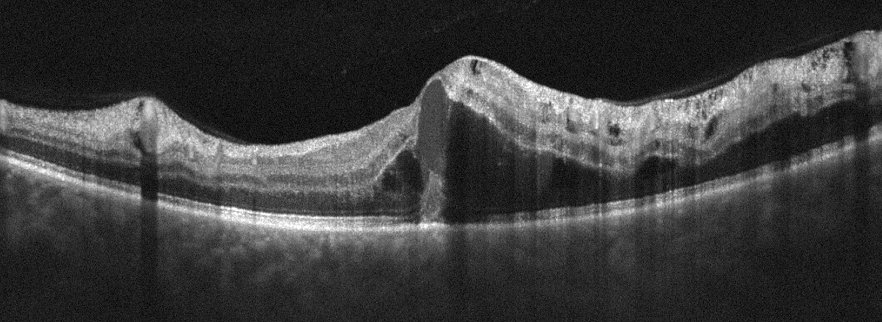
Retinal OCT cross-section. Instrument: Optovue Avanti RTVue XR
Diagnosis: retinal vein occlusion.